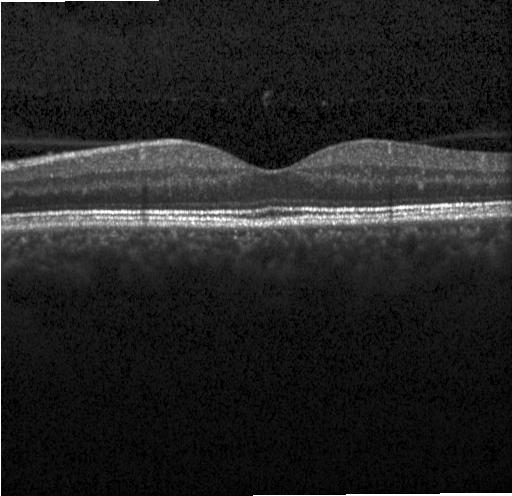

The scan shows neither CNV, DME, nor drusen.